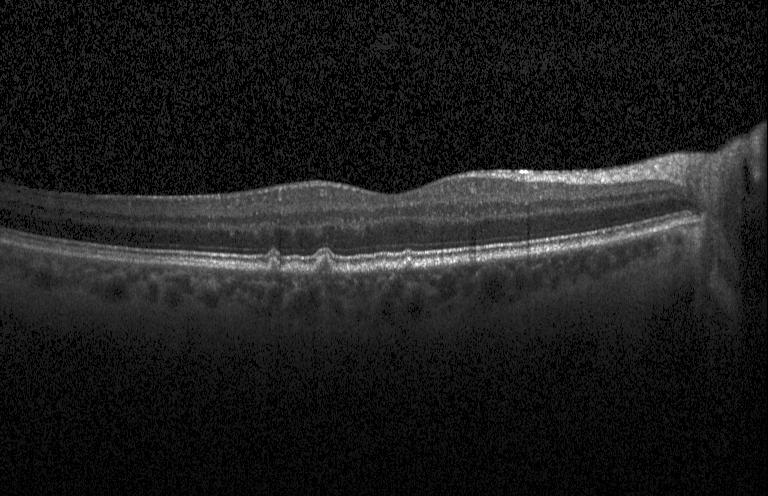
This B-scan demonstrates multiple drusen.